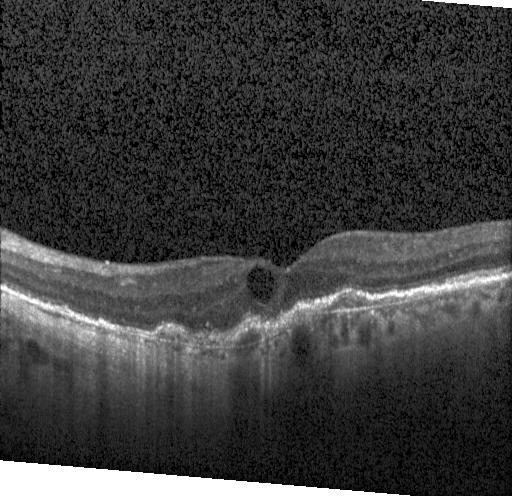

Optical coherence tomography B-scan. Spectral-domain OCT
Finding: a choroidal neovascular membrane.